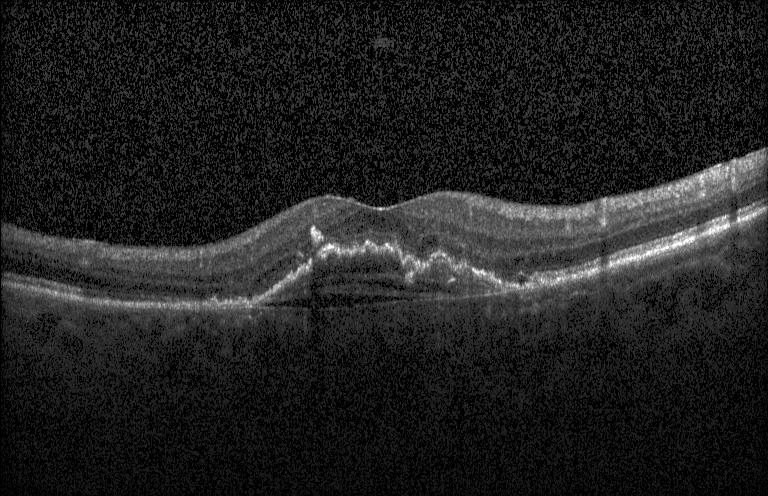

OCT B-scan
Choroidal neovascularization.